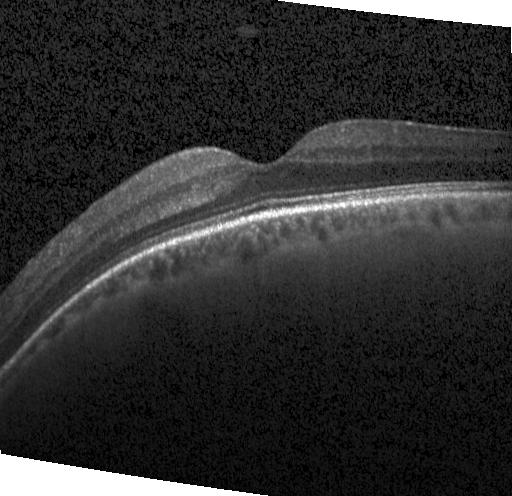
Impression: neither CNV, DME, nor drusen.